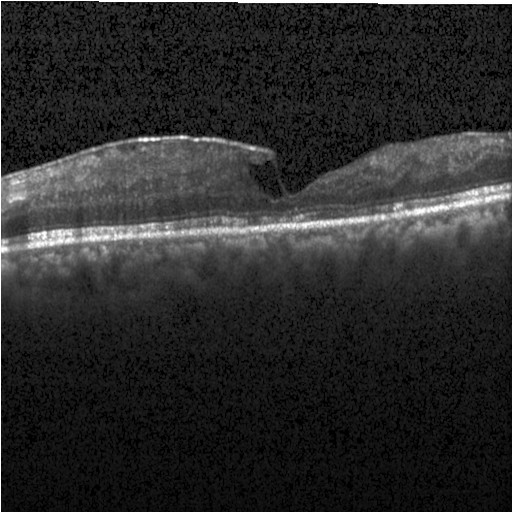 Macular OCT: DME.